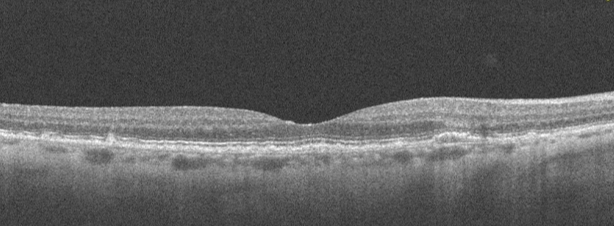
Optovue Avanti RTVue XR, retinal OCT B-scan, macular scan
OCT finding: AMD.